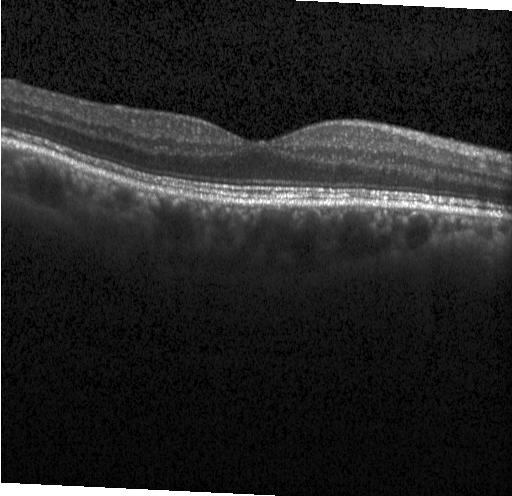

Heidelberg Spectralis OCT system; optical coherence tomography B-scan
Diagnosis: no evidence of choroidal neovascularization, diabetic macular edema, or drusen.